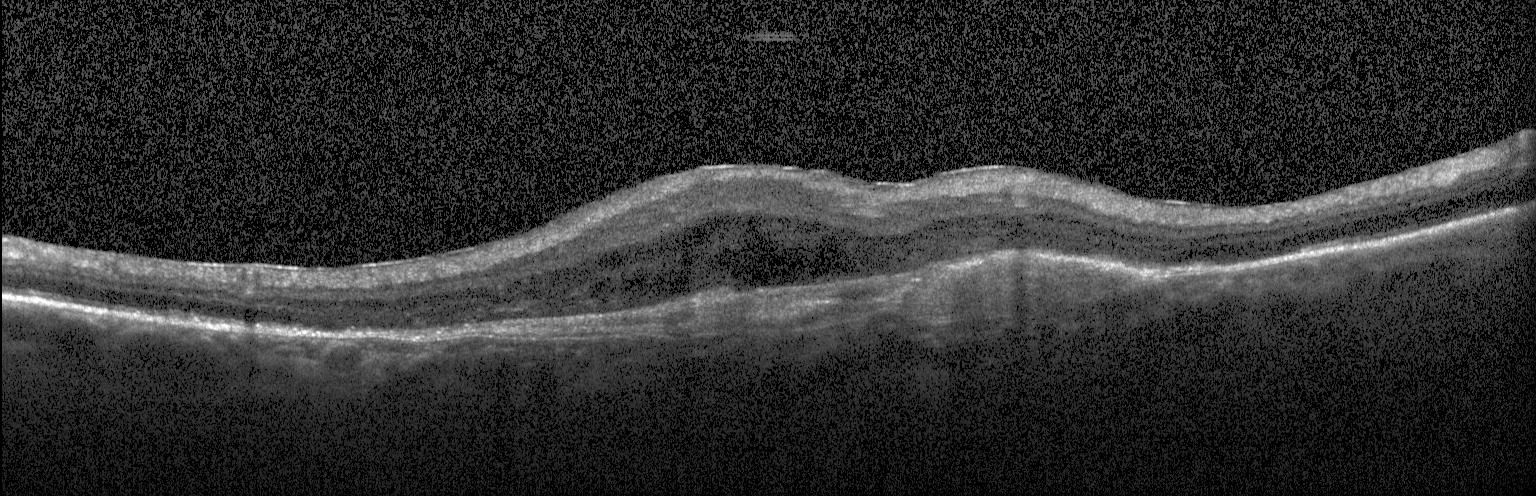 Impression: a choroidal neovascular membrane.